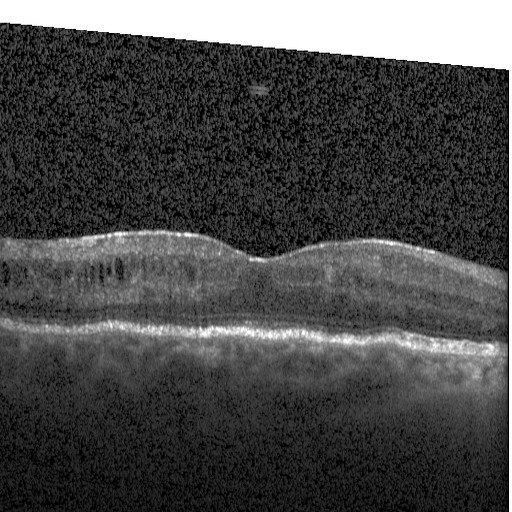

Optical coherence tomography B-scan; spectral-domain optical coherence tomography; instrument: Heidelberg Spectralis — This B-scan demonstrates diabetic macular edema.